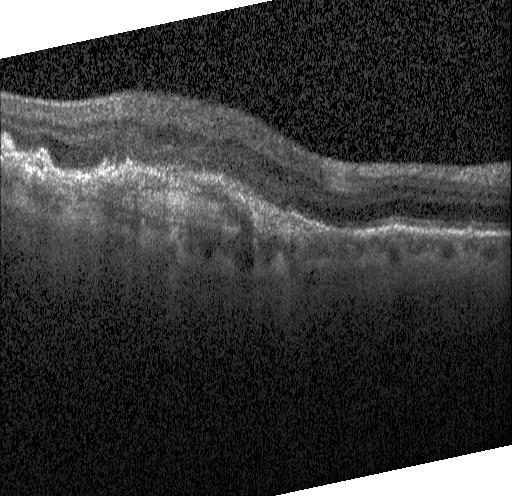

Through the macula · spectral-domain optical coherence tomography · OCT line scan · Heidelberg Spectralis. Macular OCT: a choroidal neovascular membrane.